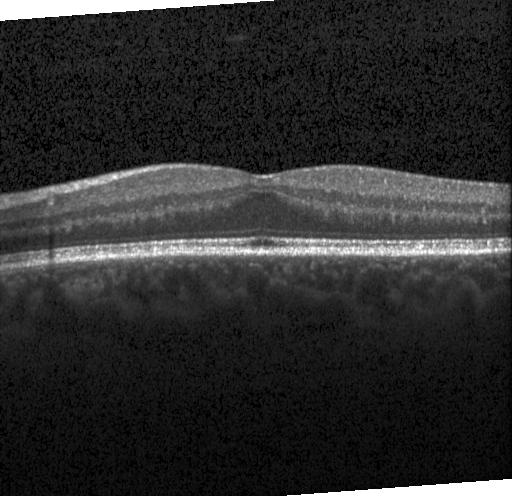

OCT B-scan. Impression: no choroidal neovascularization, no diabetic macular edema, and no drusen.